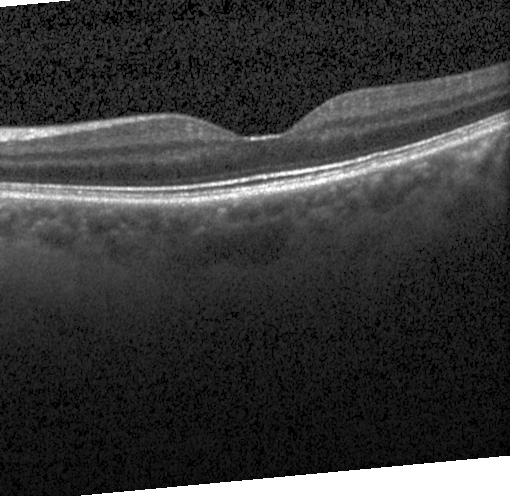

Diagnosis: neither CNV, DME, nor drusen.